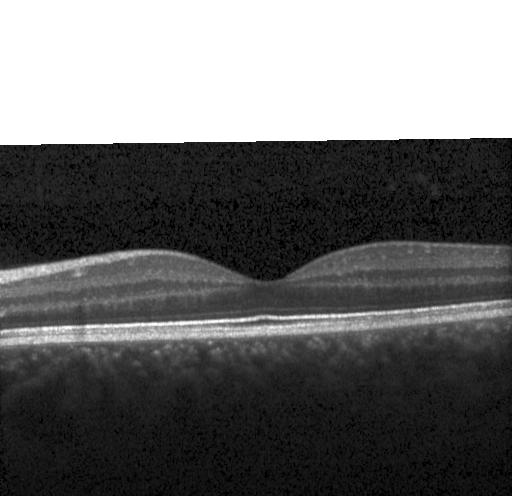

Retinal OCT cross-section; macular scan — Assessment: no evidence of choroidal neovascularization, diabetic macular edema, or drusen.